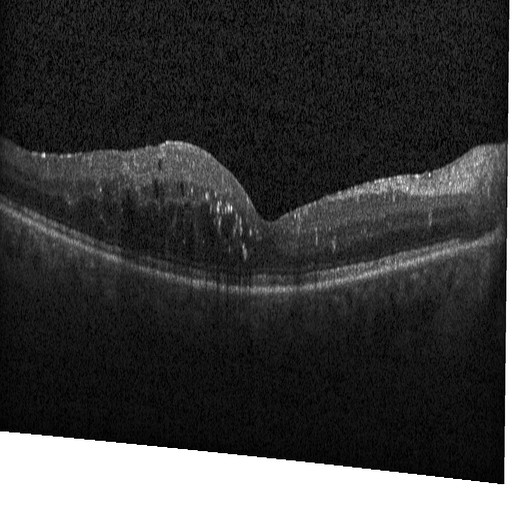

Optical coherence tomography scan. This B-scan demonstrates DME.